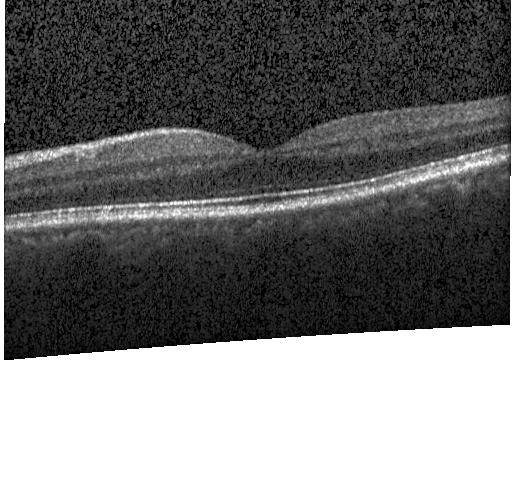
Spectral-domain optical coherence tomography, through the macula, Heidelberg Spectralis OCT system, optical coherence tomography scan. Finding: no evidence of CNV, DME, or drusen.